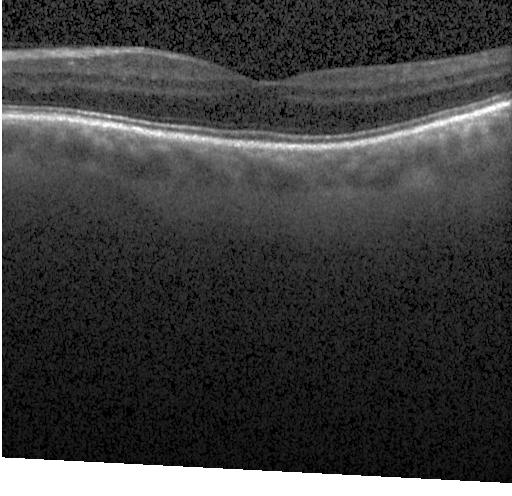
Diagnosis: no evidence of choroidal neovascularization, diabetic macular edema, or drusen.